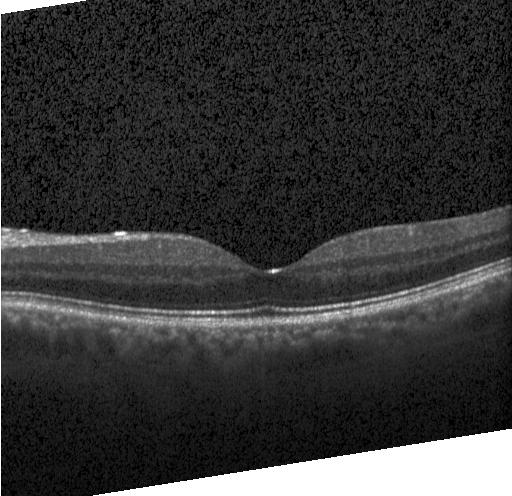

Diagnosis: no choroidal neovascularization, diabetic macular edema, or drusen.